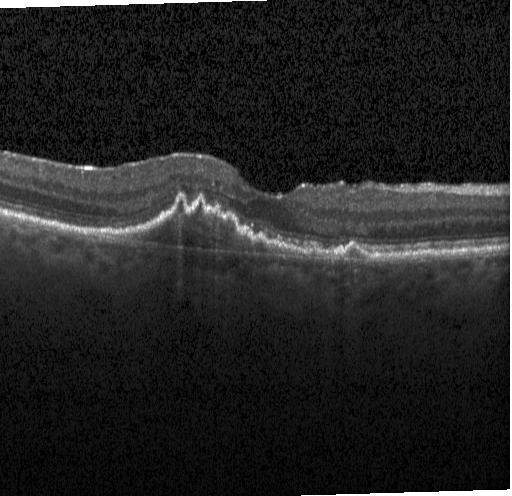

OCT line scan
Diagnosis: a choroidal neovascular membrane.